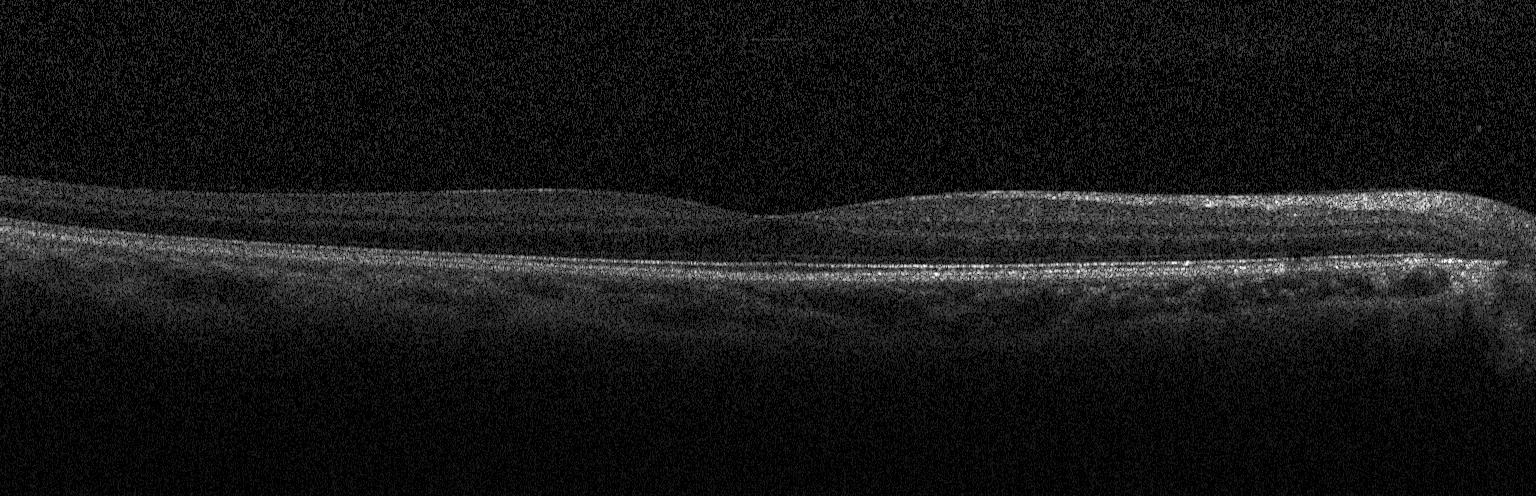

Retinal OCT cross-section. SD-OCT. Fovea-centered — Impression: neither choroidal neovascularization, diabetic macular edema, nor drusen.